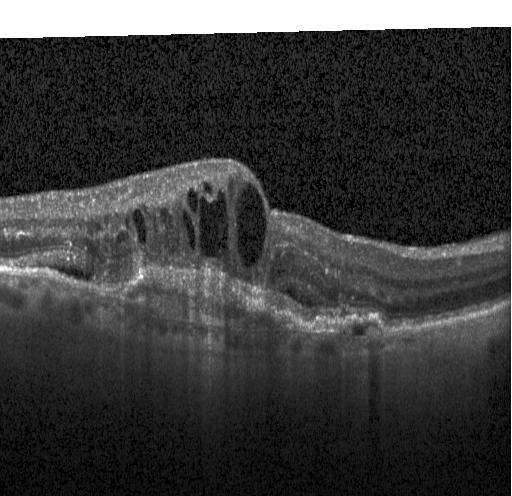
Spectral-domain OCT B-scan: choroidal neovascularization.